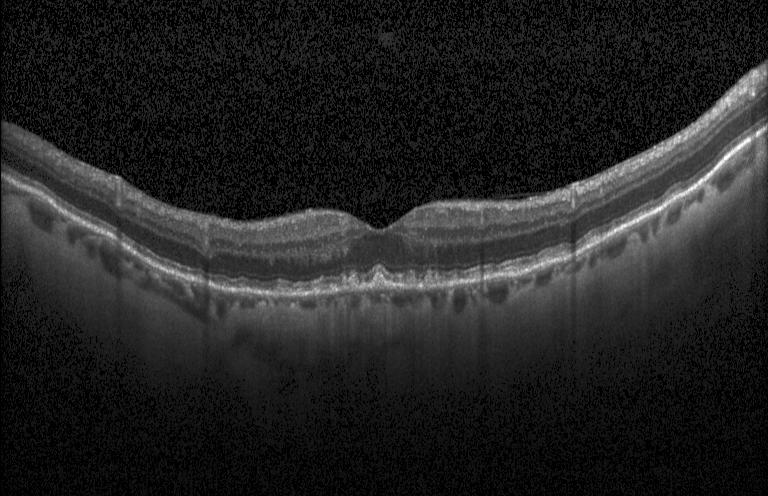

The scan shows sub-RPE drusenoid deposits.